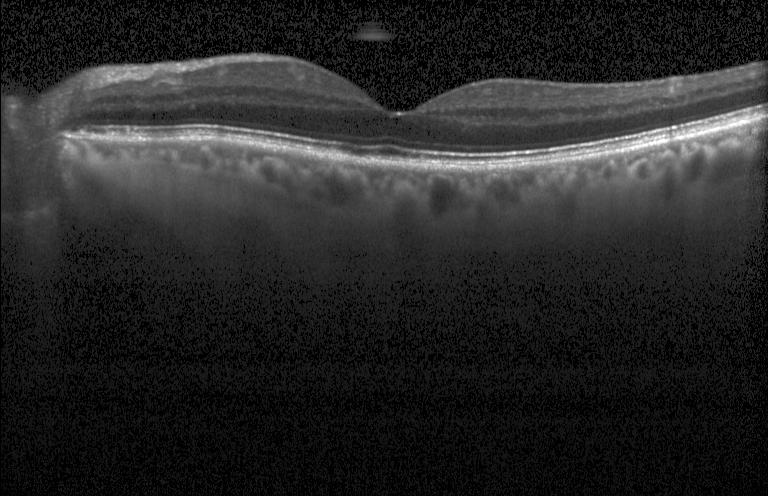
Fovea-centered. OCT B-scan — No choroidal neovascularization, diabetic macular edema, or drusen.